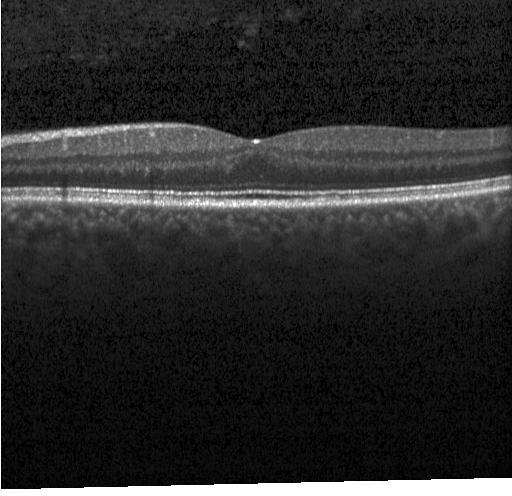

Optical coherence tomography B-scan; spectral-domain optical coherence tomography.
This B-scan demonstrates neither CNV, DME, nor drusen.